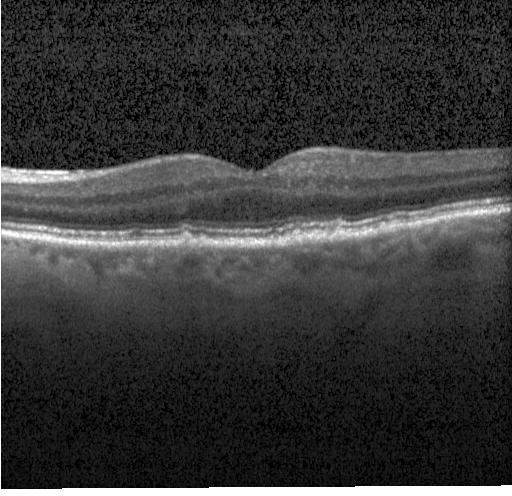 OCT line scan
This B-scan demonstrates multiple drusen.